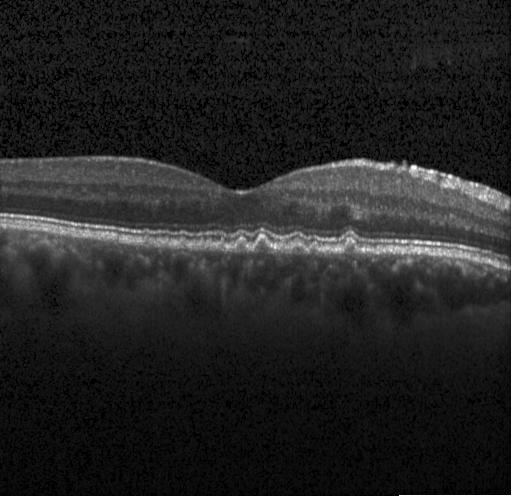 OCT B-scan; Heidelberg Spectralis OCT system.
Diagnosis: sub-RPE drusenoid deposits.